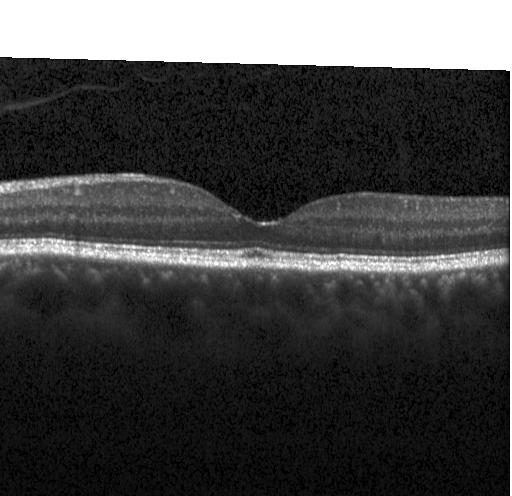
Retinal OCT B-scan, SD-OCT, instrument: Heidelberg Spectralis, fovea-centered
This B-scan demonstrates no choroidal neovascularization, no diabetic macular edema, and no drusen.